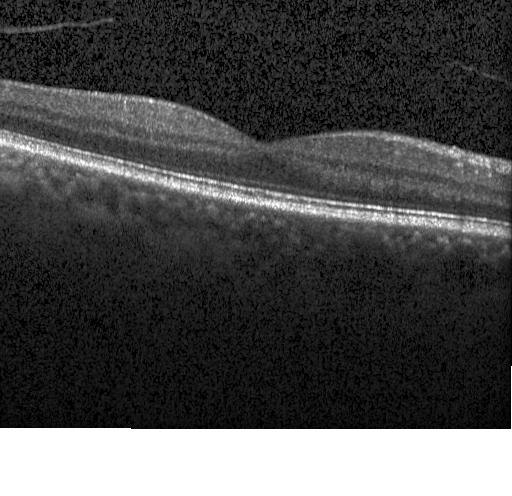

Fovea-centered. OCT B-scan — Macular OCT: neither choroidal neovascularization, diabetic macular edema, nor drusen.